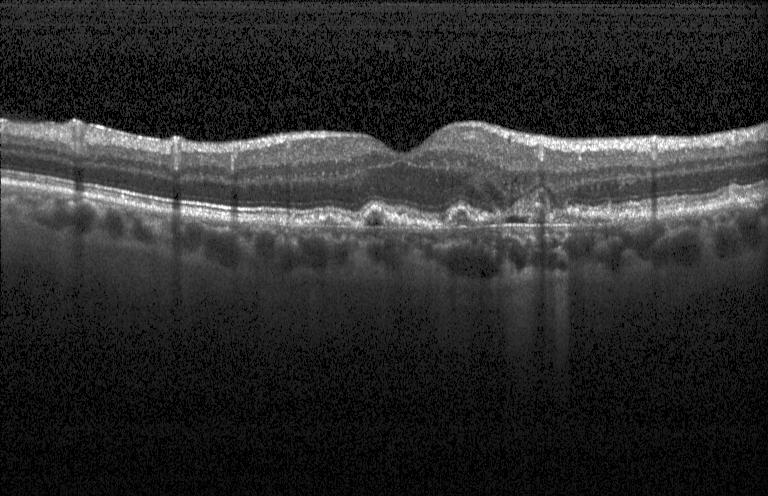 Fovea-centered, optical coherence tomography B-scan. The scan shows sub-RPE drusenoid deposits.